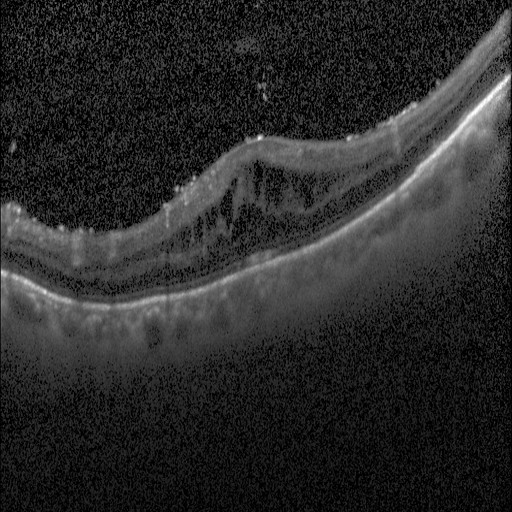

OCT line scan, macular scan, spectral-domain optical coherence tomography, Heidelberg Spectralis — Impression: diabetic macular edema.